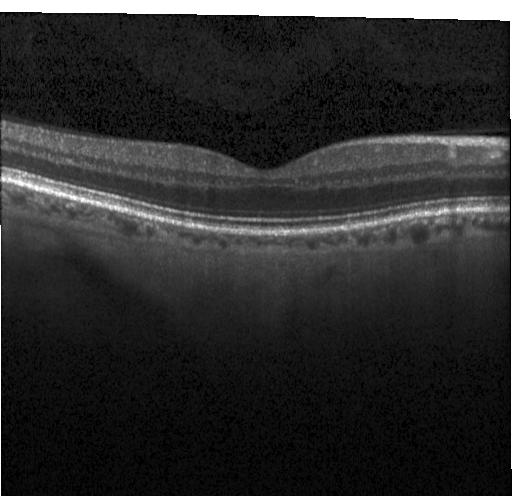

Impression: no evidence of choroidal neovascularization, diabetic macular edema, or drusen.